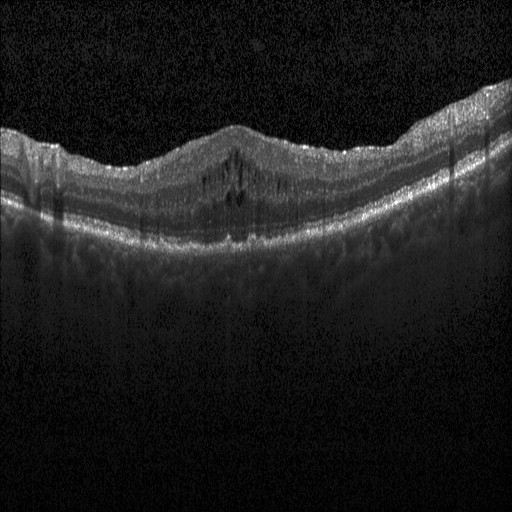

Heidelberg Spectralis · retinal OCT cross-section · macular scan — Impression: DME.